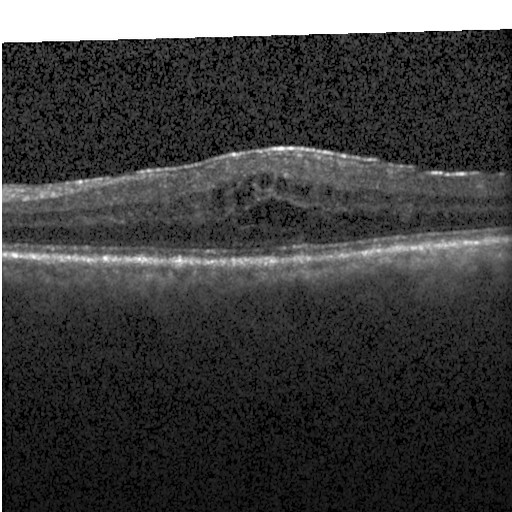

Spectral-domain optical coherence tomography · macular scan · OCT B-scan
Finding: DME.